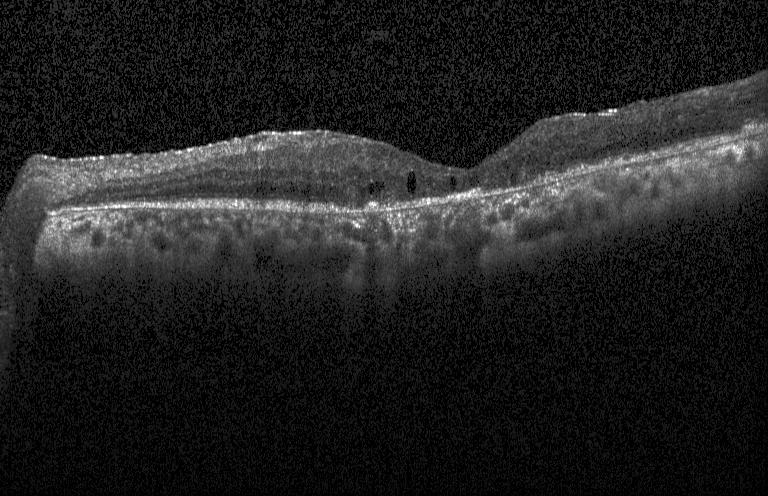

Through the macula. Spectral-domain OCT. Retinal OCT B-scan. Diagnosis: choroidal neovascularization.